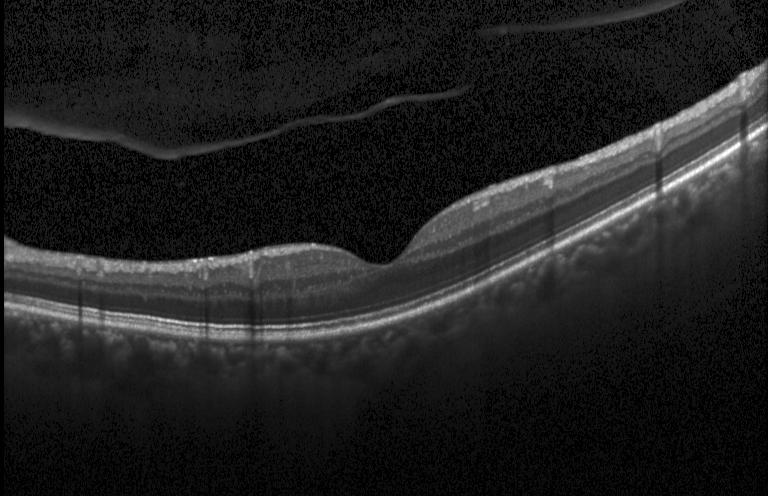

Retinal OCT cross-section. Diagnosis: no choroidal neovascularization, diabetic macular edema, or drusen.